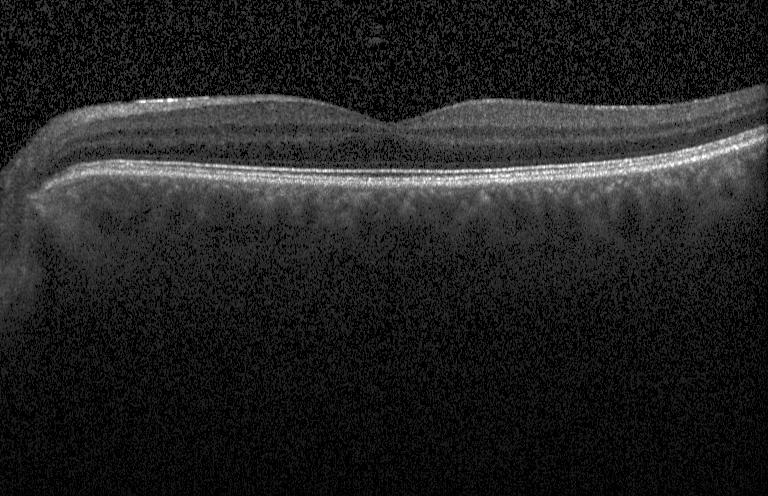
Impression: no evidence of choroidal neovascularization, diabetic macular edema, or drusen.